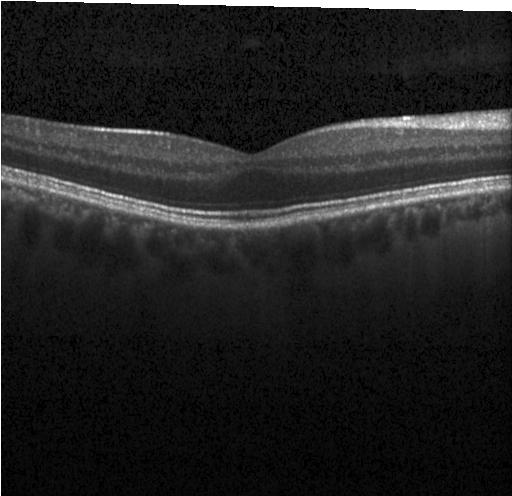

Heidelberg Spectralis; retinal OCT cross-section — Impression: no choroidal neovascularization, diabetic macular edema, or drusen.